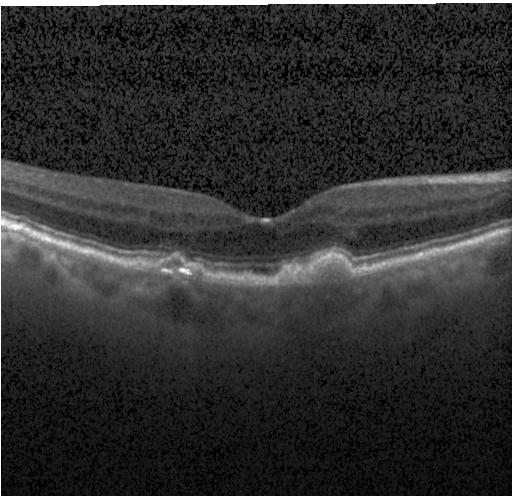 Impression: multiple drusen.